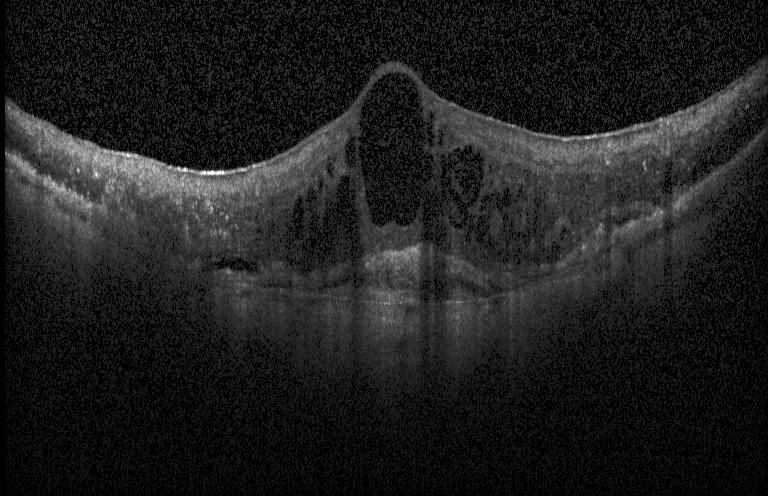 Macular scan. Optical coherence tomography scan. Spectral-domain OCT. Acquired on a Heidelberg Spectralis.
OCT finding: choroidal neovascularization.